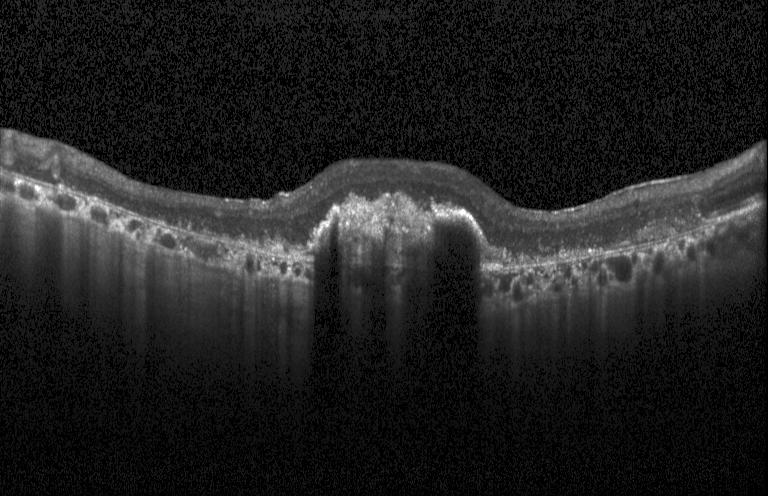 Instrument: Heidelberg Spectralis · SD-OCT · OCT B-scan · centered on the fovea
Assessment: choroidal neovascularization (CNV).